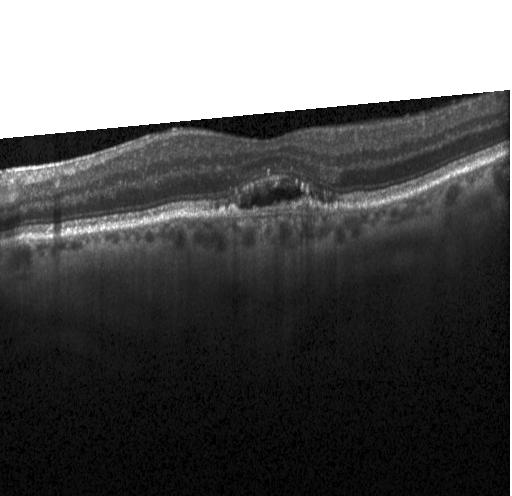 Instrument: Heidelberg Spectralis; retinal OCT cross-section; spectral-domain OCT
Macular OCT: a choroidal neovascular membrane.